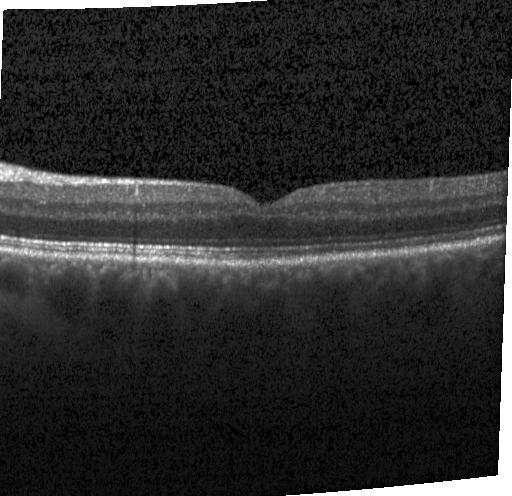
Optical coherence tomography B-scan — Dx: neither choroidal neovascularization, diabetic macular edema, nor drusen.